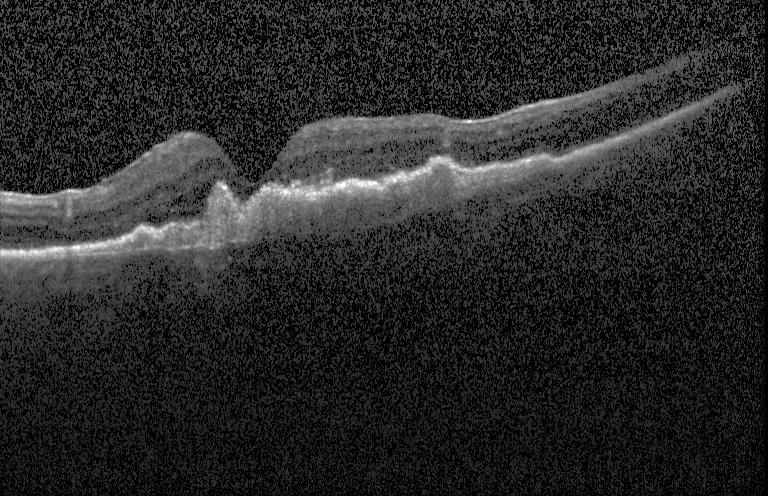 Centered on the fovea · retinal OCT B-scan
This B-scan demonstrates choroidal neovascularization (CNV).